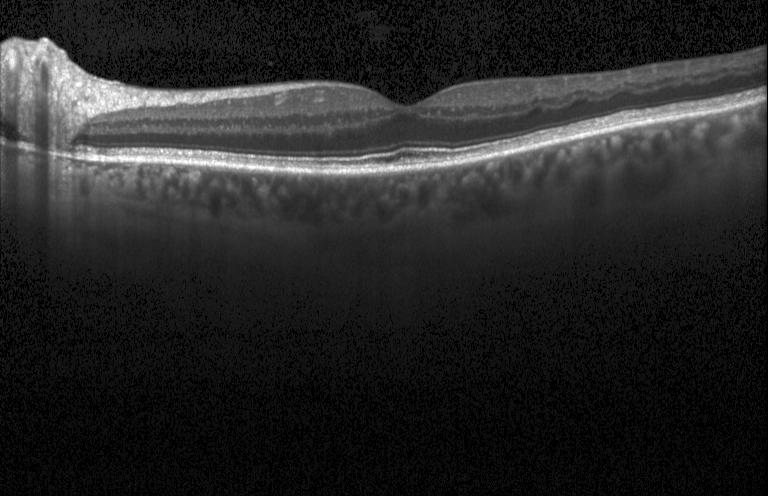 Finding: no CNV, no DME, and no drusen.